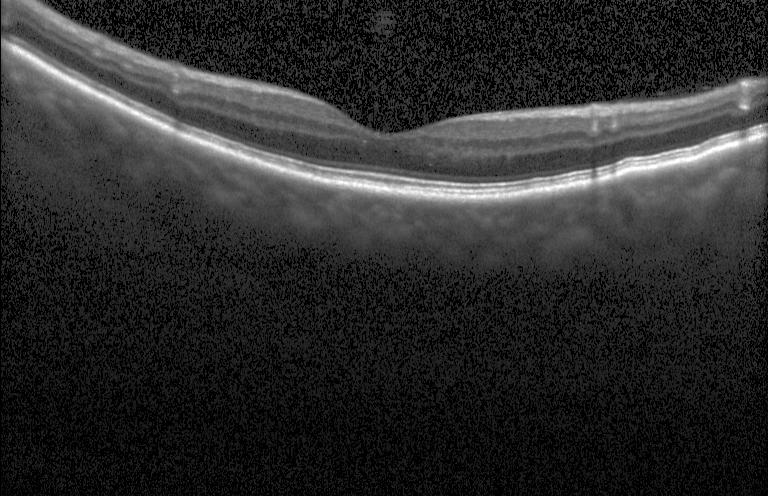
Impression: neither choroidal neovascularization, diabetic macular edema, nor drusen.